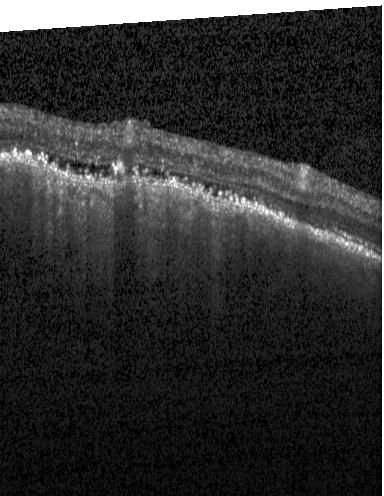

Retinal OCT B-scan. This B-scan demonstrates CNV.